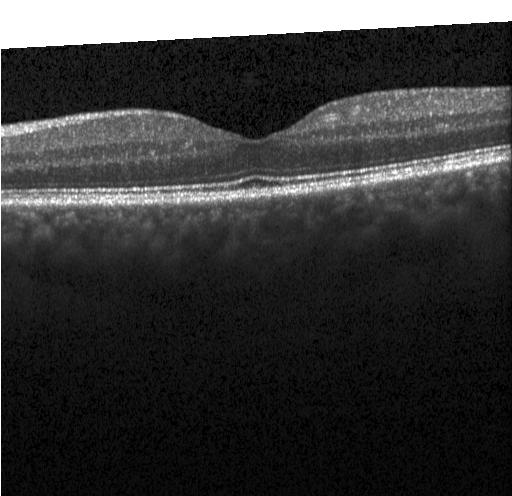 OCT finding: no CNV, no DME, and no drusen.